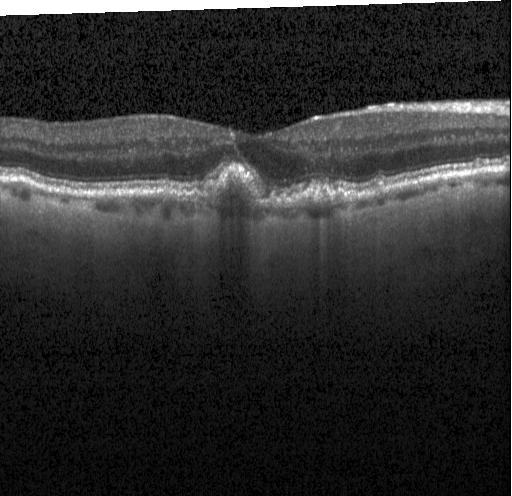

OCT line scan
Assessment: multiple drusen.